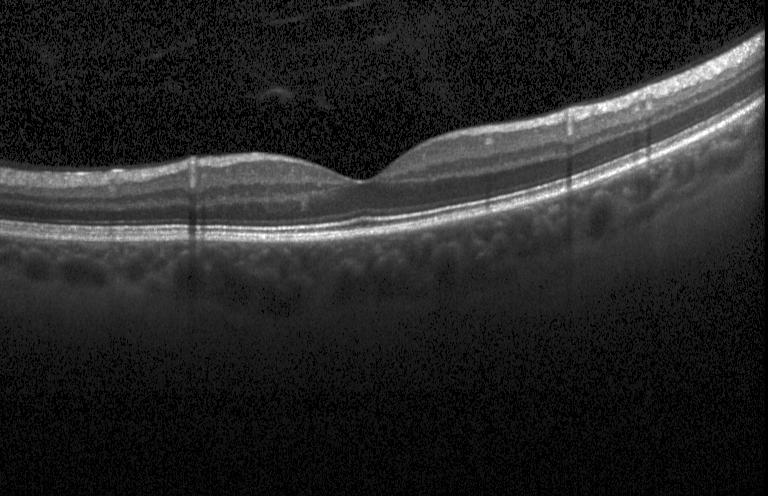
OCT line scan. Spectral-domain OCT. Impression: neither choroidal neovascularization, diabetic macular edema, nor drusen.